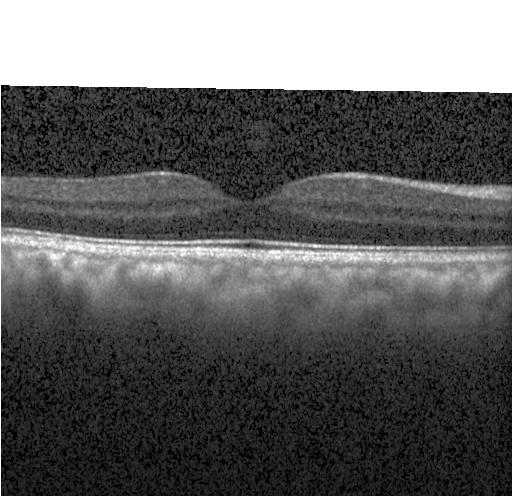 OCT B-scan. Acquired on a Heidelberg Spectralis. Through the macula. SD-OCT. OCT finding: neither choroidal neovascularization, diabetic macular edema, nor drusen.